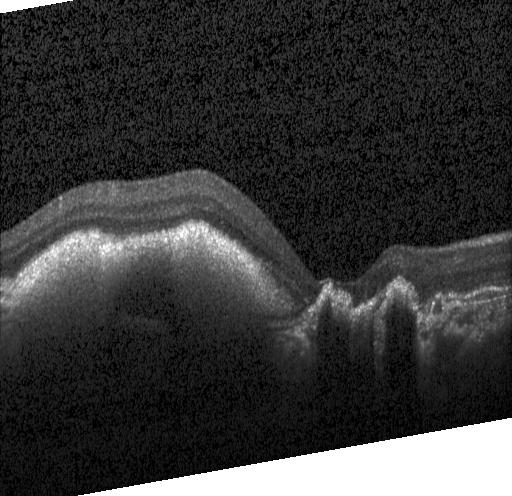 Finding: a choroidal neovascular membrane.